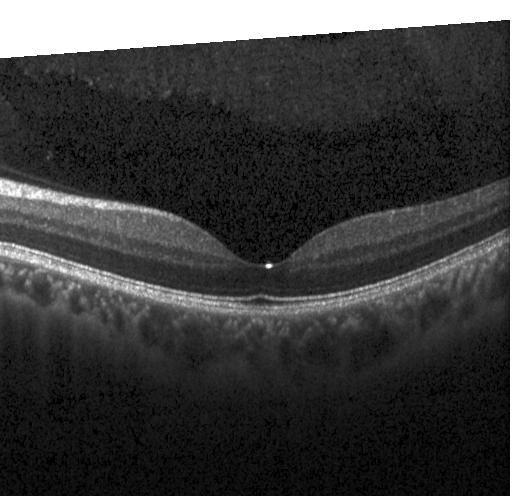

SD-OCT; optical coherence tomography B-scan; through the macula. Finding: no evidence of choroidal neovascularization, diabetic macular edema, or drusen.